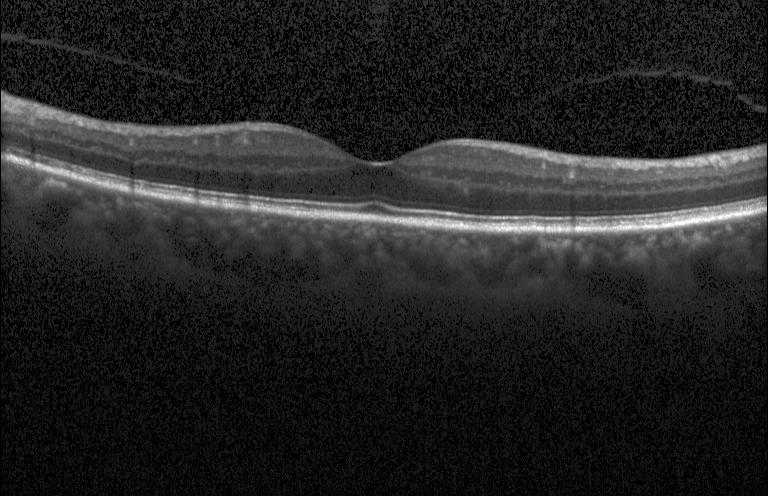

Heidelberg Spectralis, macular scan, SD-OCT, OCT B-scan. Impression: neither choroidal neovascularization, diabetic macular edema, nor drusen.